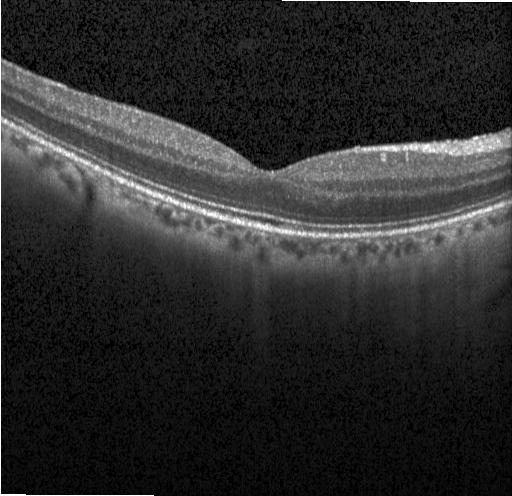 SD-OCT, OCT line scan, through the macula. Diagnosis: neither choroidal neovascularization, diabetic macular edema, nor drusen.